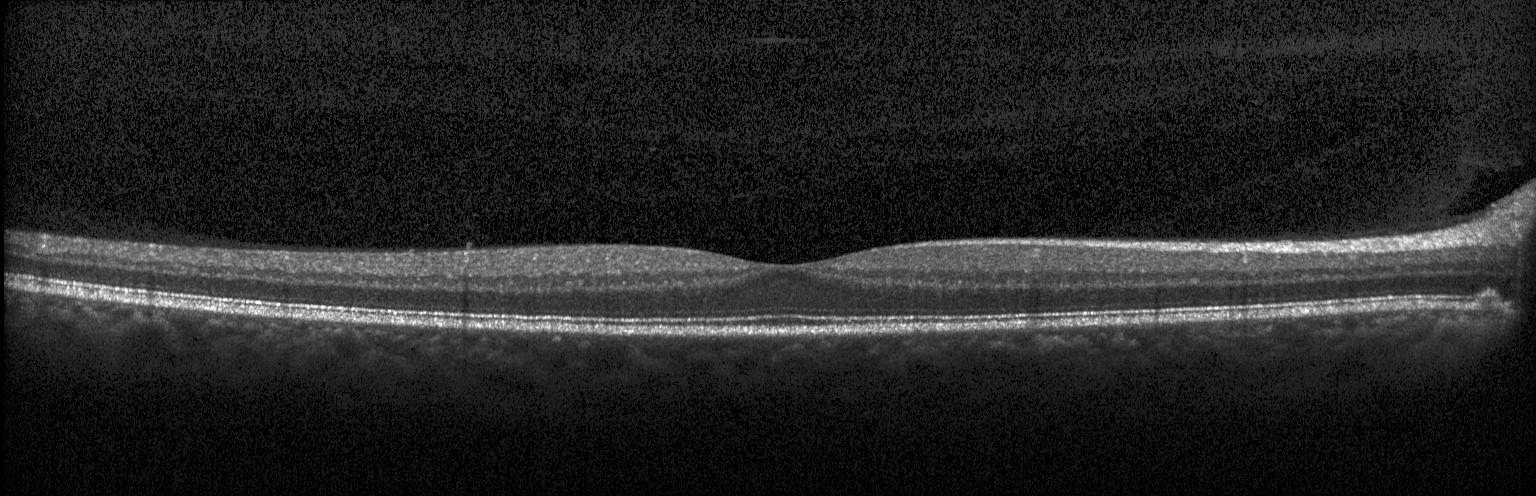
Dx: neither choroidal neovascularization, diabetic macular edema, nor drusen.